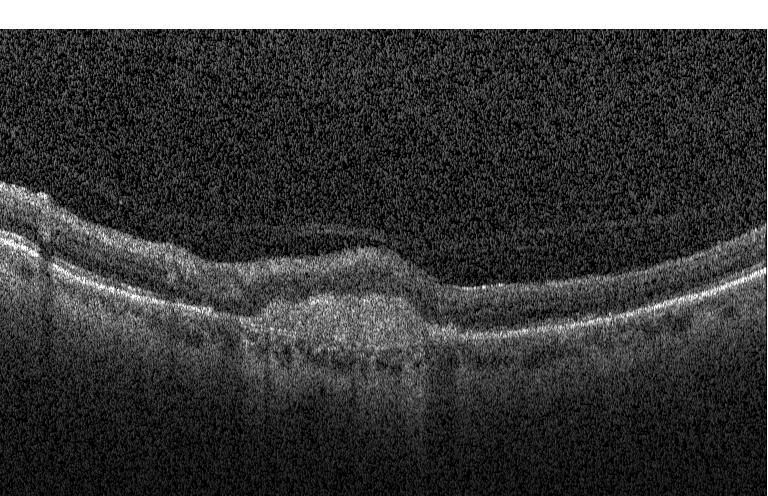
Impression: choroidal neovascularization.